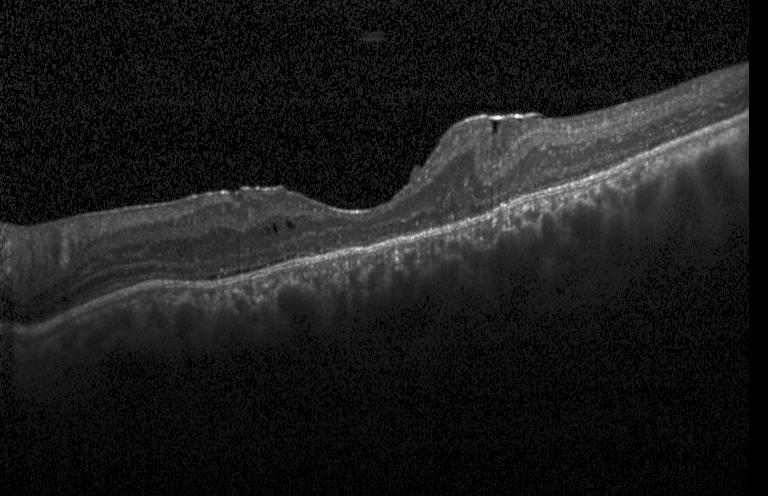
Assessment: diabetic macular edema (DME).